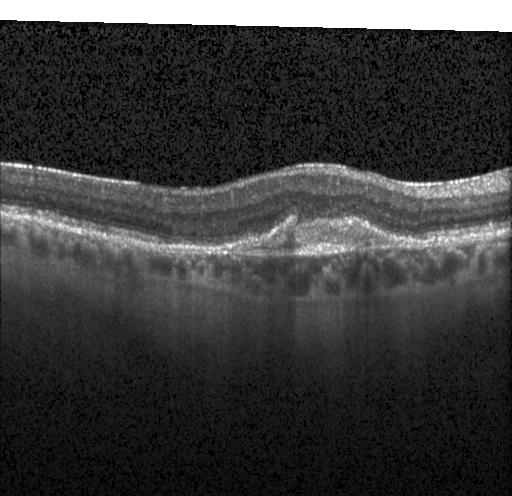

Heidelberg Spectralis. OCT line scan — Macular OCT: choroidal neovascularization (CNV).